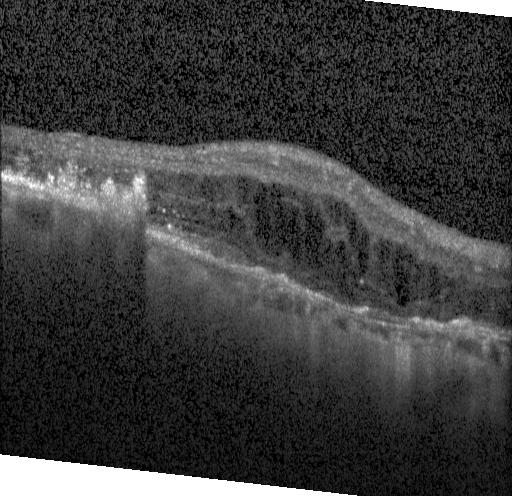
Finding: CNV.